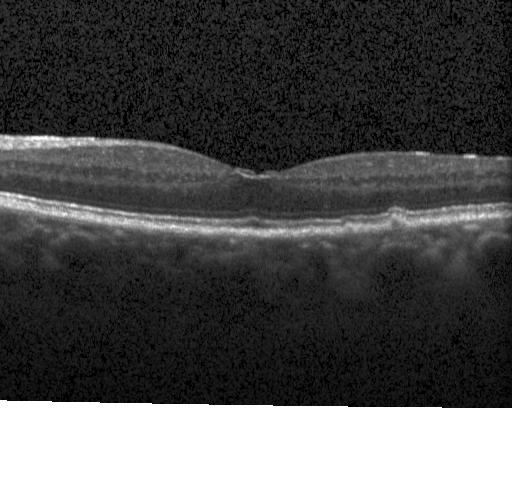
Impression: multiple drusen.